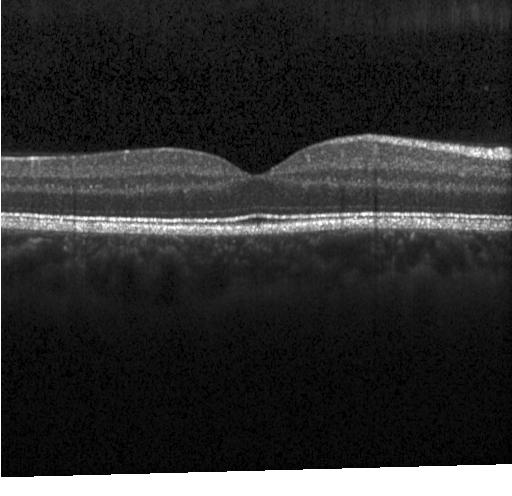

Finding: neither choroidal neovascularization, diabetic macular edema, nor drusen.